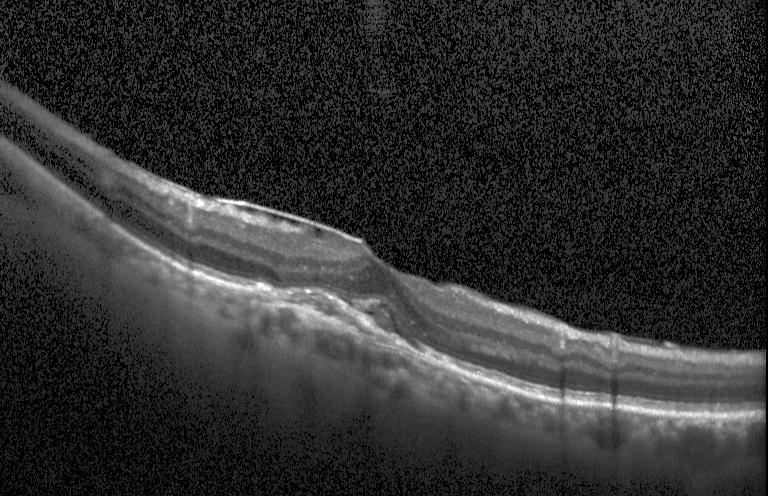 Spectral-domain OCT, OCT B-scan, through the macula — Finding: a choroidal neovascular membrane.